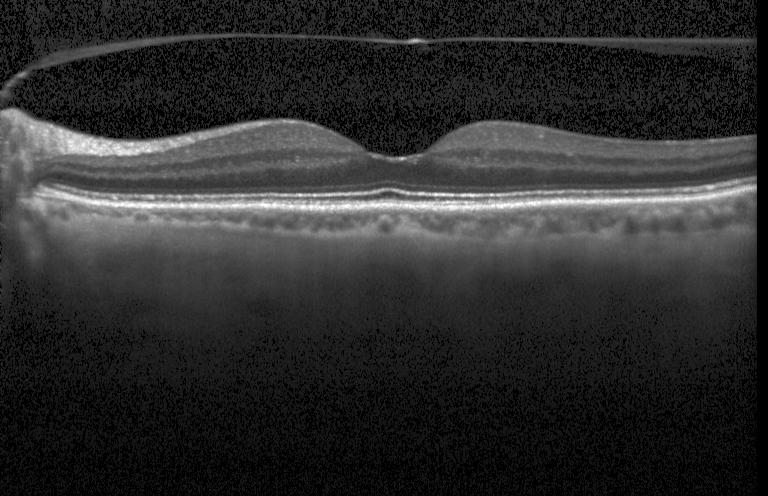 Spectral-domain OCT B-scan: no CNV, no DME, and no drusen.